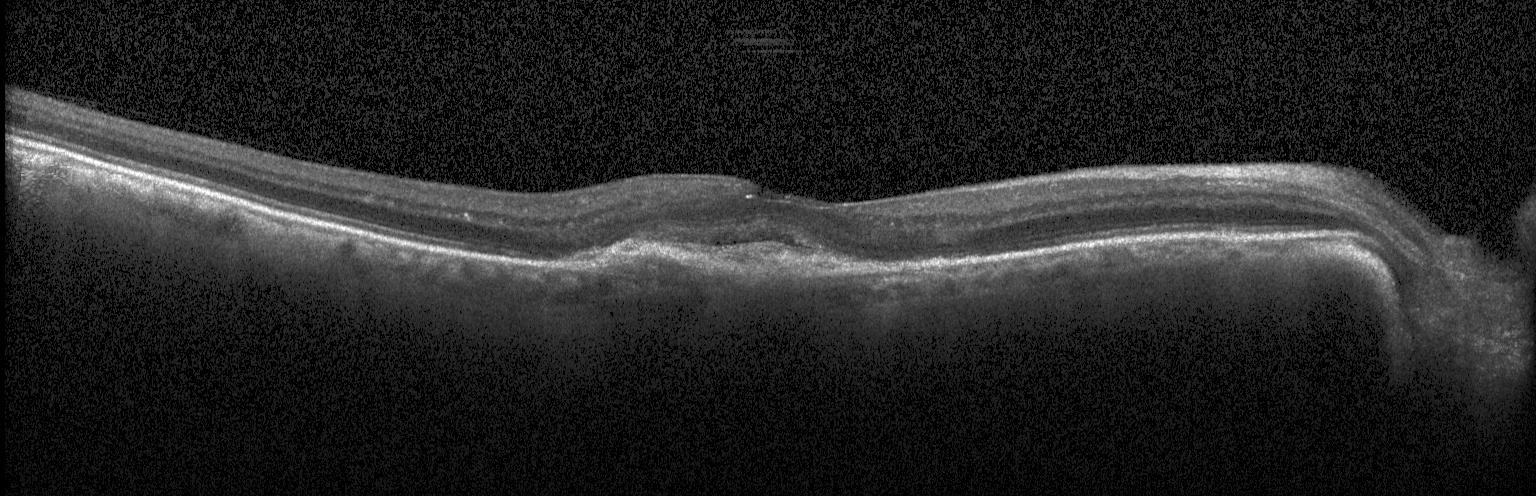
Macular OCT: choroidal neovascularization.